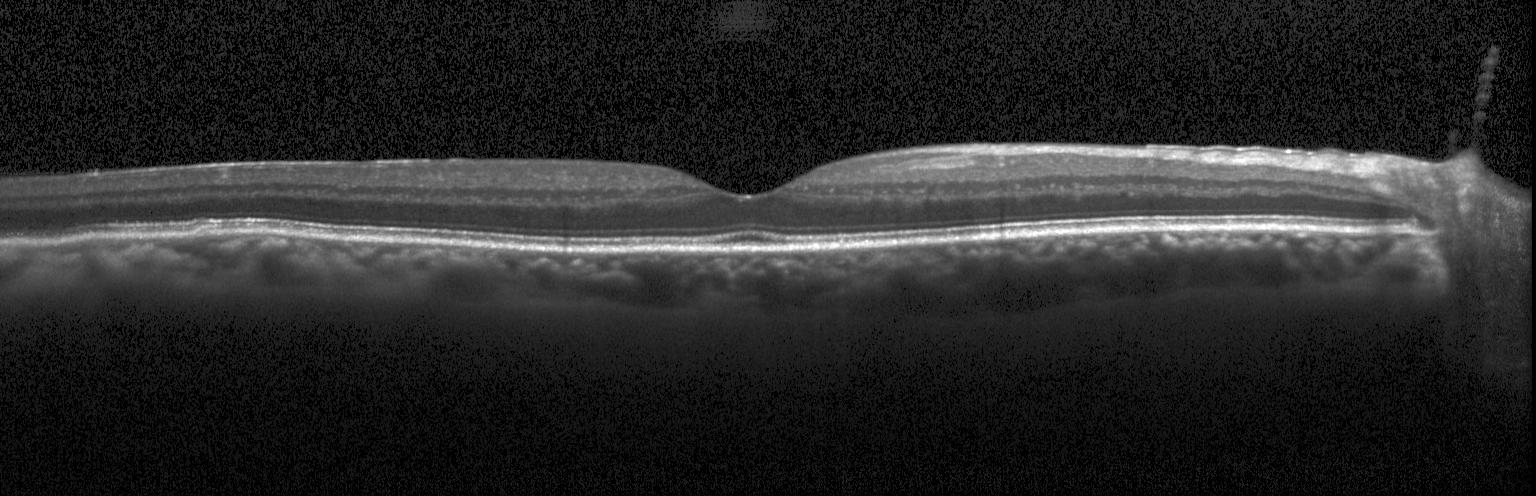

Through the macula; optical coherence tomography scan; Heidelberg Spectralis OCT system.
Assessment: neither choroidal neovascularization, diabetic macular edema, nor drusen.